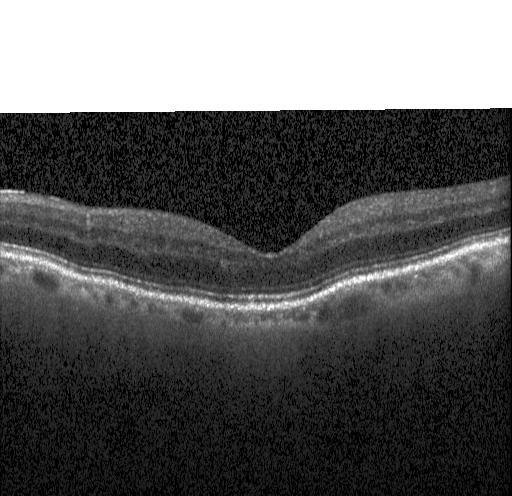

Dx: neither CNV, DME, nor drusen.